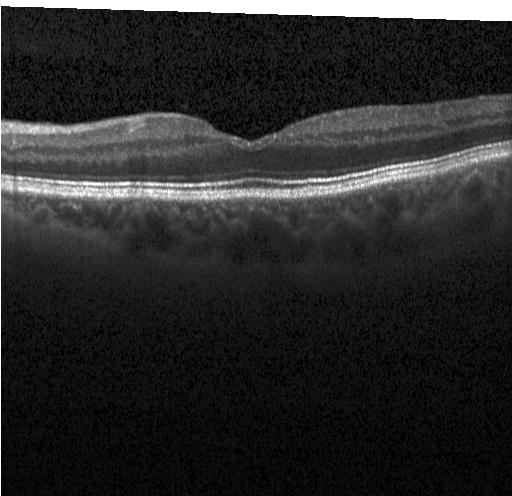
Optical coherence tomography B-scan. Finding: neither choroidal neovascularization, diabetic macular edema, nor drusen.